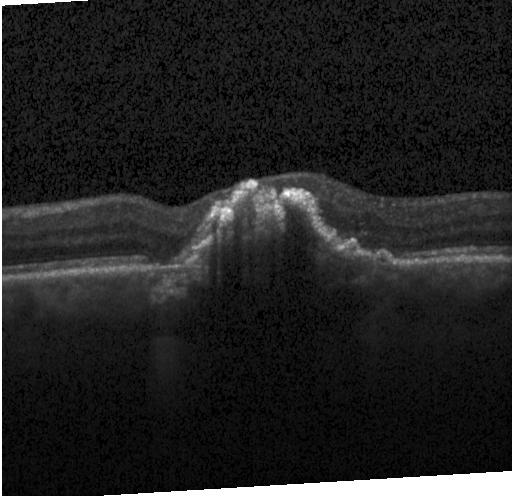
Spectral-domain optical coherence tomography. Heidelberg Spectralis OCT system. Retinal OCT cross-section
Impression: a choroidal neovascular membrane.